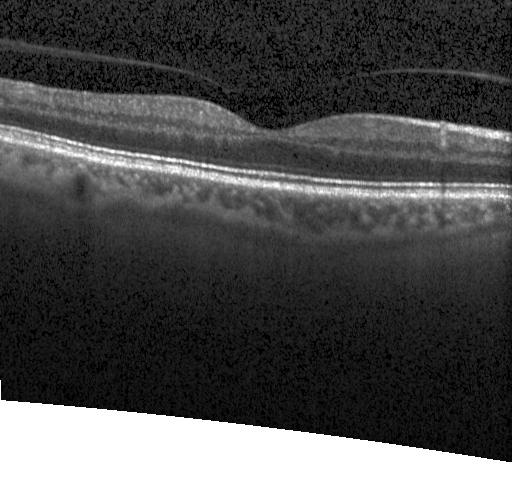

Heidelberg Spectralis OCT system, centered on the fovea, optical coherence tomography scan, spectral-domain optical coherence tomography.
Impression: neither choroidal neovascularization, diabetic macular edema, nor drusen.